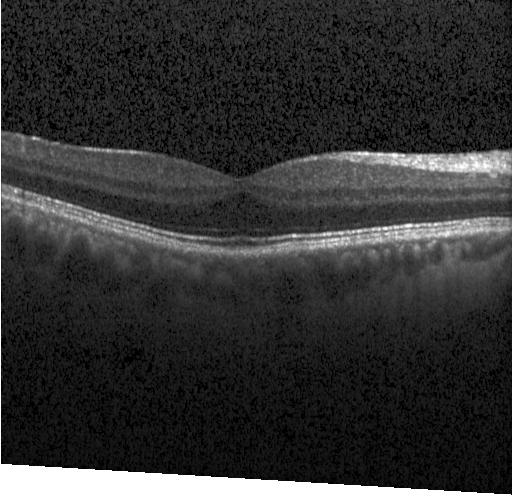

Macular OCT: no evidence of CNV, DME, or drusen.